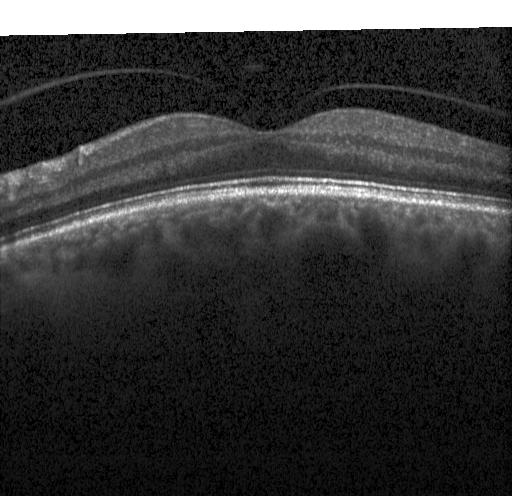

The scan shows neither choroidal neovascularization, diabetic macular edema, nor drusen.